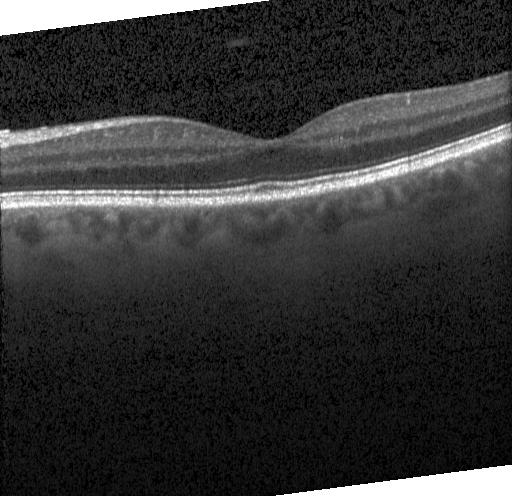 OCT B-scan · Heidelberg Spectralis OCT system. Finding: no choroidal neovascularization, no diabetic macular edema, and no drusen.